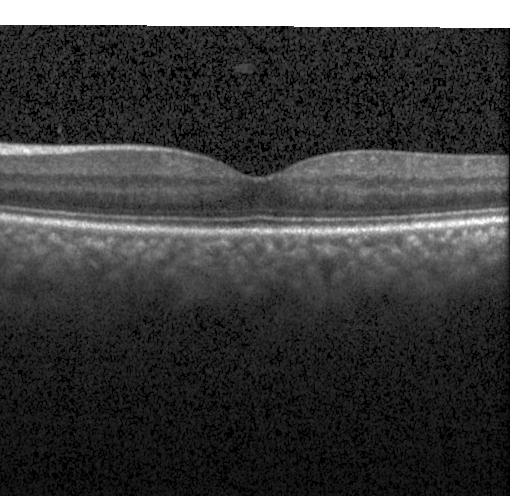 Acquired on a Heidelberg Spectralis, OCT B-scan, spectral-domain OCT, horizontal scan through the fovea
Finding: no choroidal neovascularization, no diabetic macular edema, and no drusen.